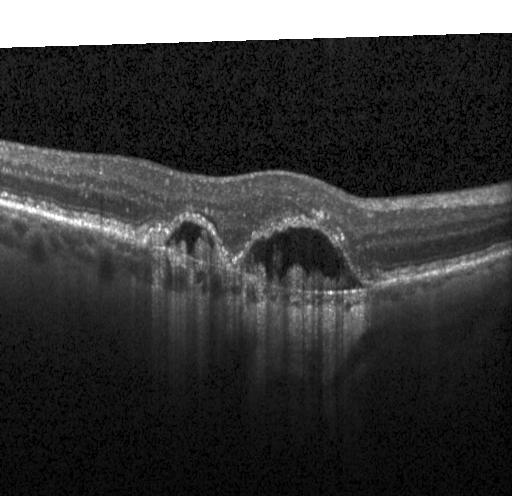 Fovea-centered; OCT line scan.
Finding: a choroidal neovascular membrane.